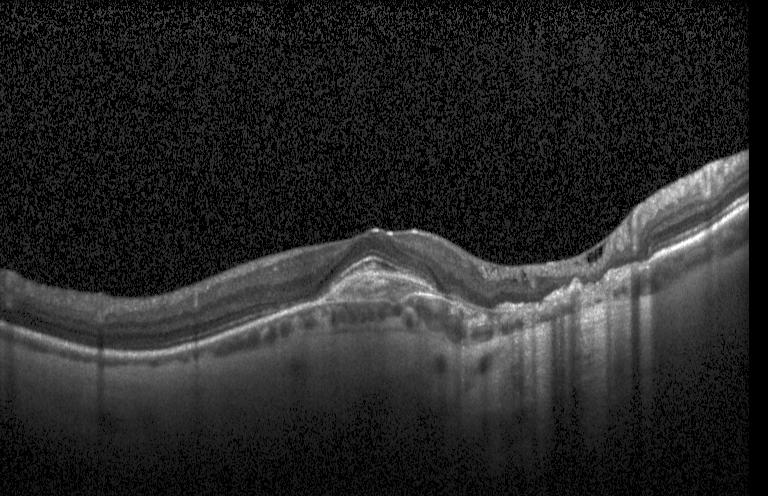
Retinal OCT cross-section showing choroidal neovascularization.